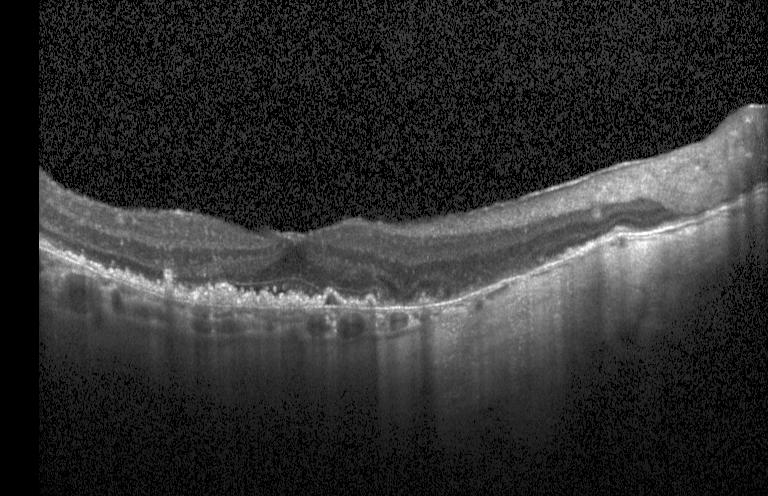 Choroidal neovascularization (CNV).